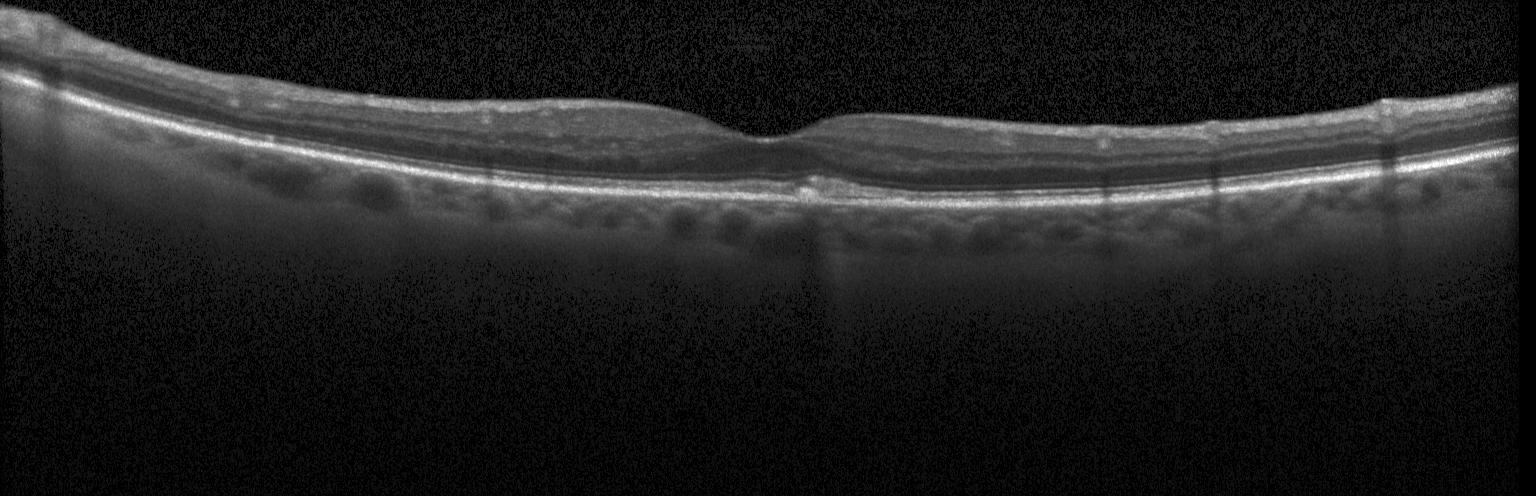

OCT B-scan, through the macula, spectral-domain OCT. Finding: multiple drusen.